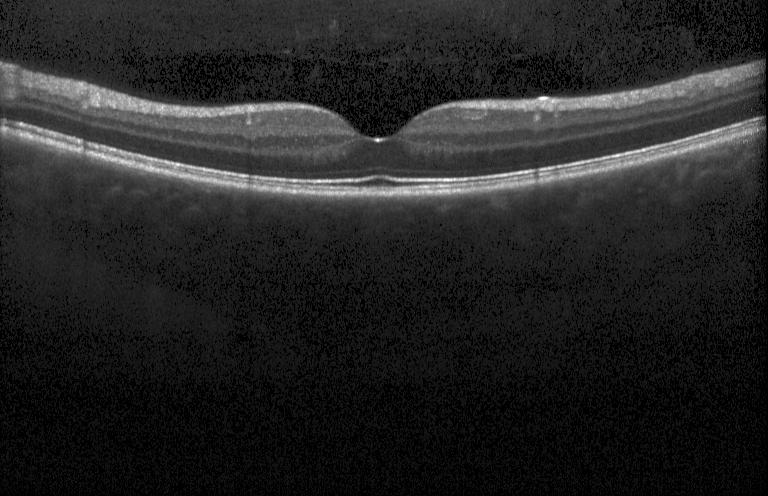 Macular OCT: no evidence of choroidal neovascularization, diabetic macular edema, or drusen.